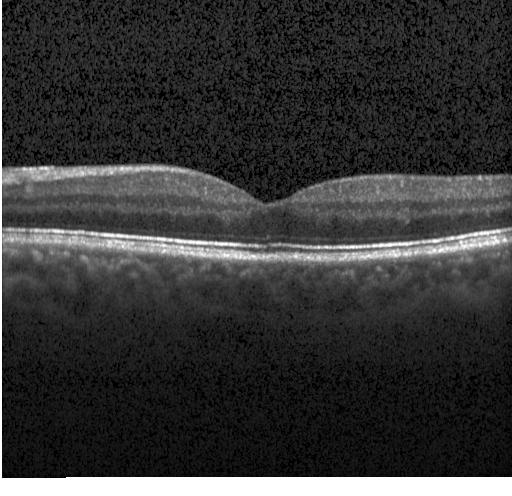 Neither choroidal neovascularization, diabetic macular edema, nor drusen.